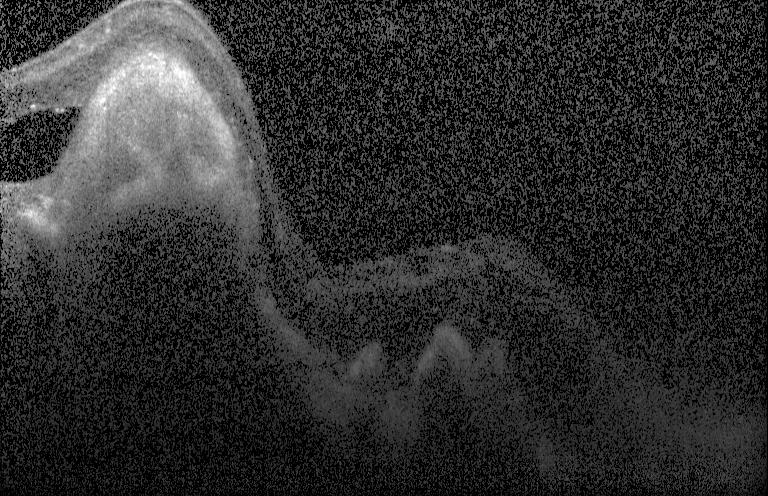

OCT B-scan — Impression: CNV.